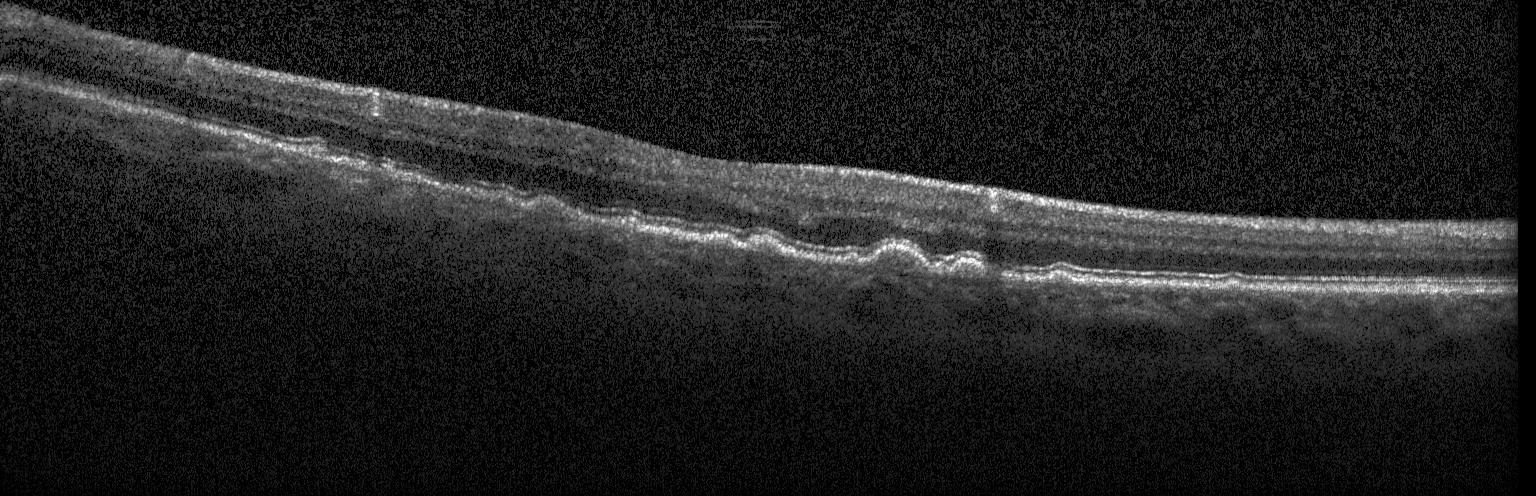
OCT B-scan · Heidelberg Spectralis.
This B-scan demonstrates multiple drusen.